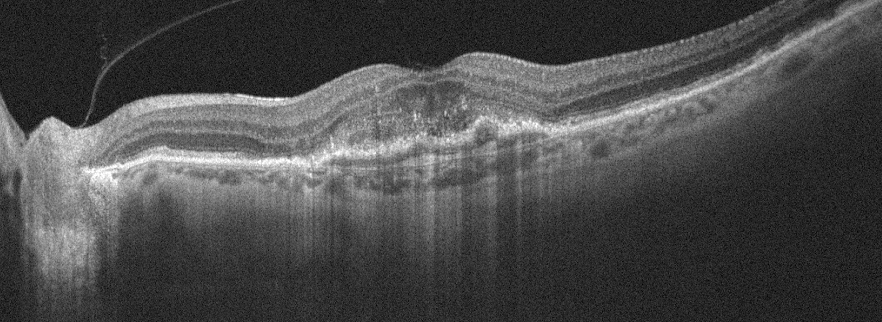

Left eye. Retinal OCT B-scan — AMD.